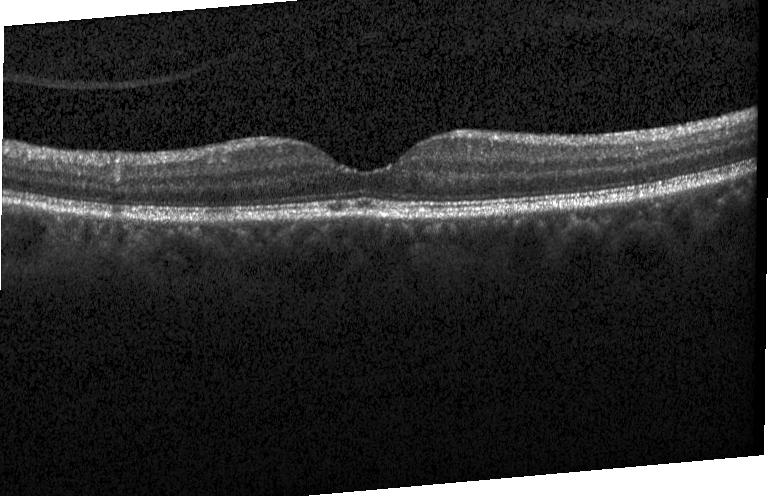 Heidelberg Spectralis OCT system, horizontal scan through the fovea, spectral-domain OCT, OCT line scan. Finding: no evidence of choroidal neovascularization, diabetic macular edema, or drusen.